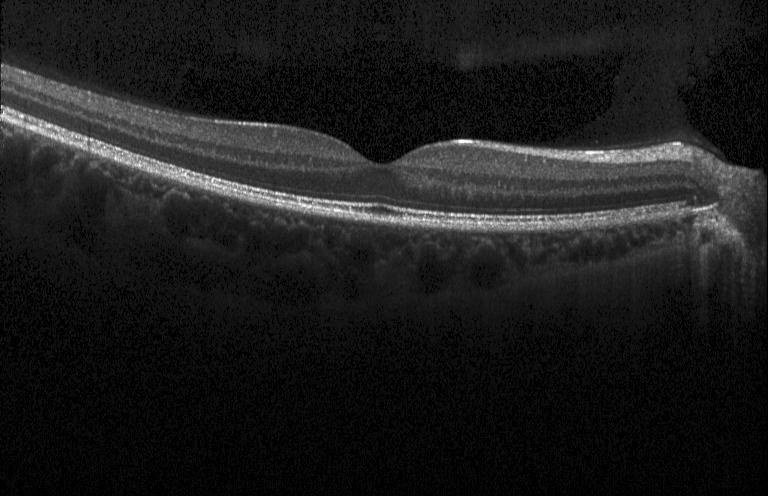

Macular OCT: neither CNV, DME, nor drusen.